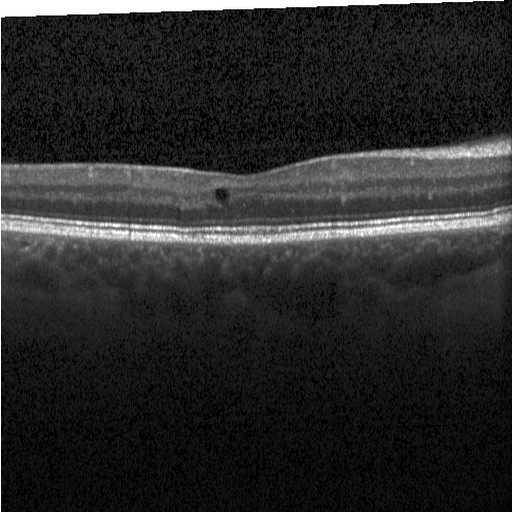 Retinal OCT B-scan; horizontal scan through the fovea; acquired on a Heidelberg Spectralis — Diagnosis: diabetic macular edema (DME).